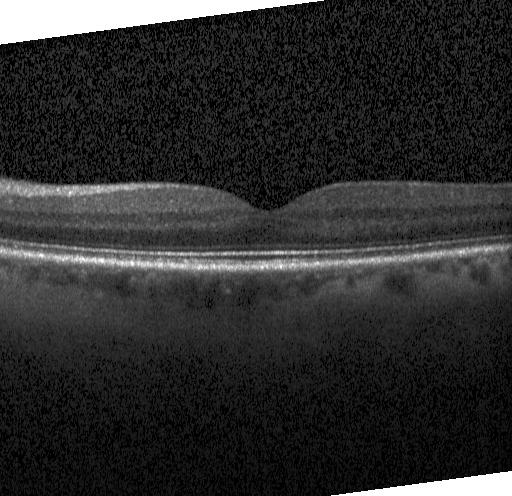 OCT B-scan showing neither CNV, DME, nor drusen.